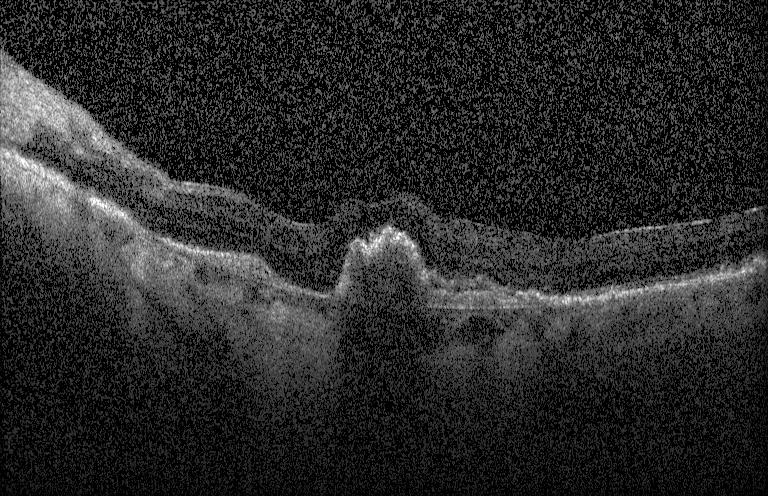 Optical coherence tomography B-scan. The scan shows CNV.